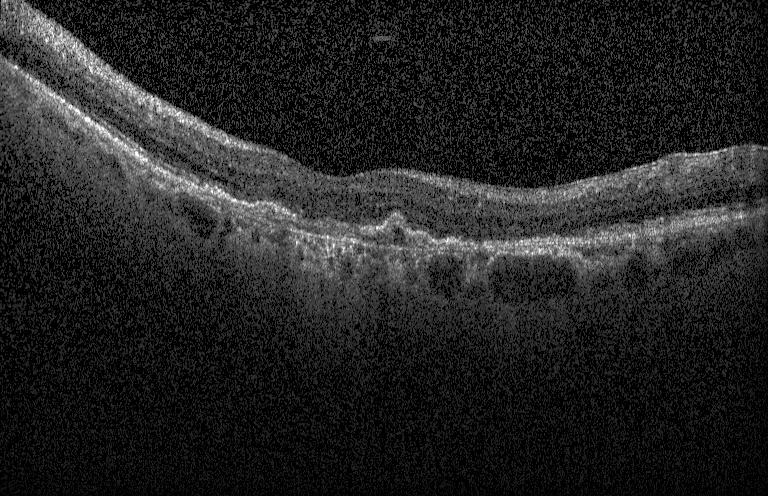

Instrument: Heidelberg Spectralis; optical coherence tomography scan. Impression: a choroidal neovascular membrane.